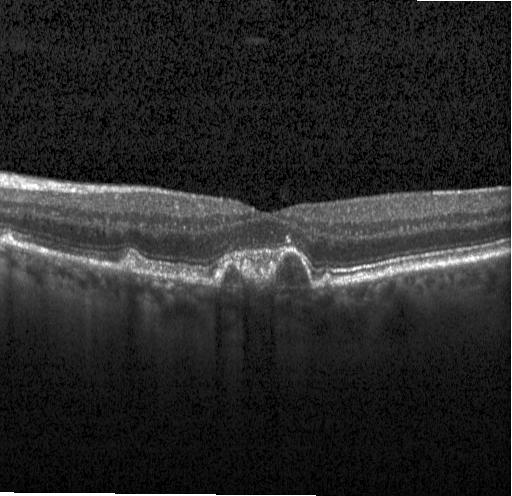
Centered on the fovea; OCT B-scan — OCT finding: CNV.